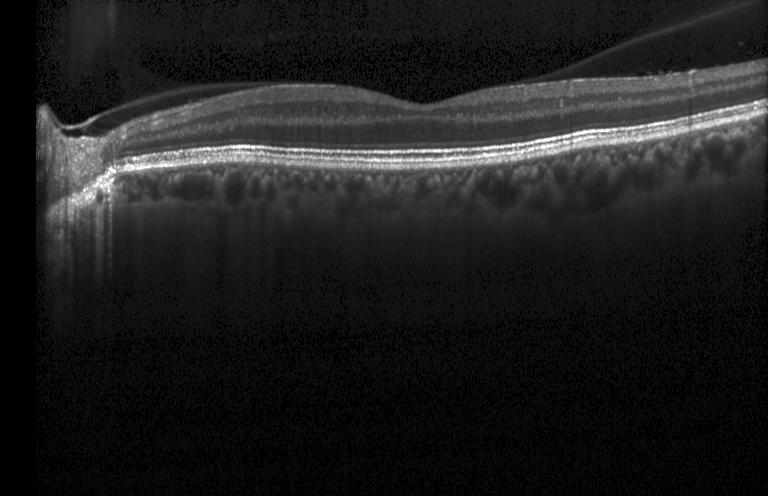

Spectral-domain OCT. Heidelberg Spectralis. Horizontal scan through the fovea. OCT line scan.
Impression: neither CNV, DME, nor drusen.